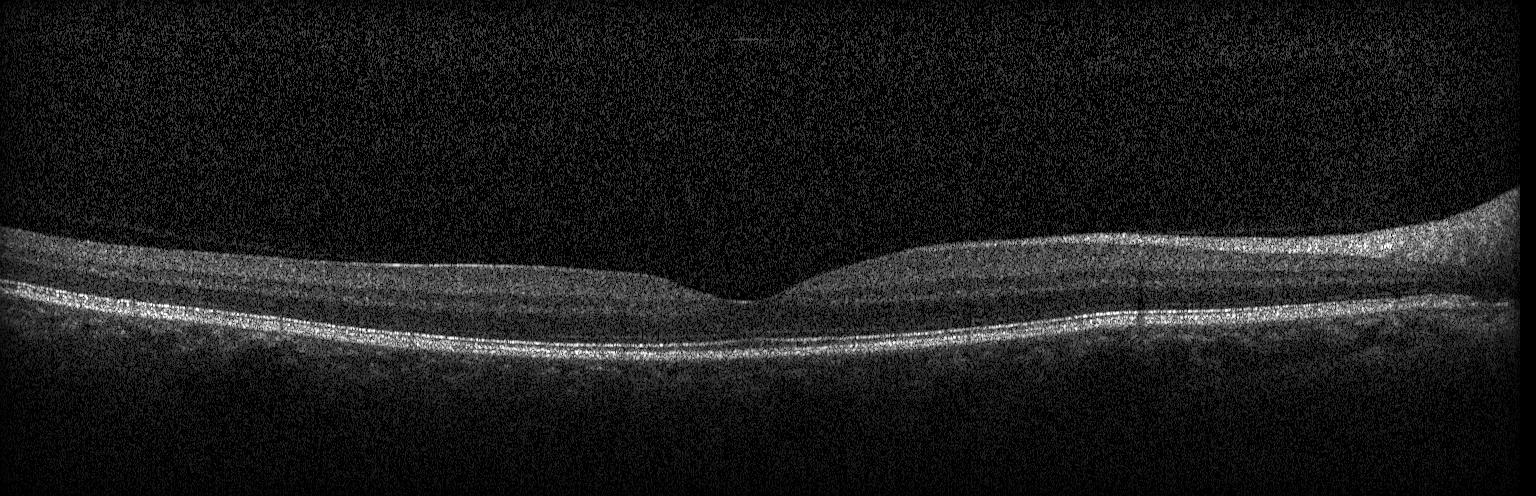
Horizontal scan through the fovea, Heidelberg Spectralis OCT system, retinal OCT B-scan
Finding: no choroidal neovascularization, no diabetic macular edema, and no drusen.